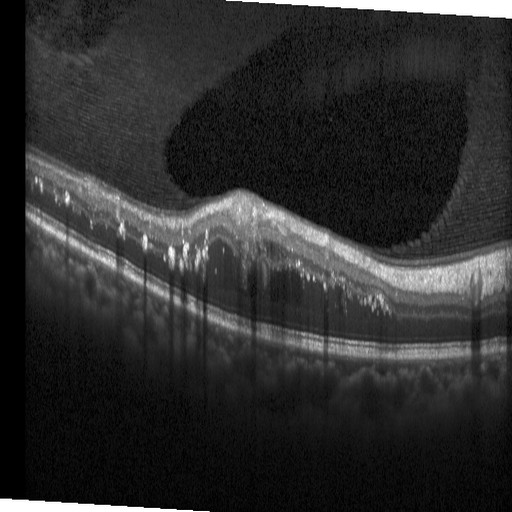

Macular OCT: diabetic macular edema (DME).